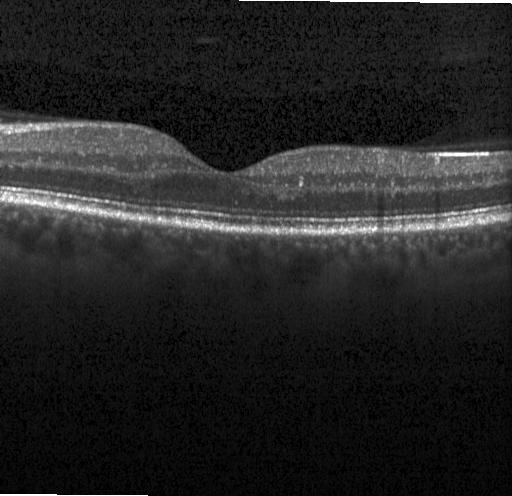 OCT B-scan.
Diagnosis: neither choroidal neovascularization, diabetic macular edema, nor drusen.